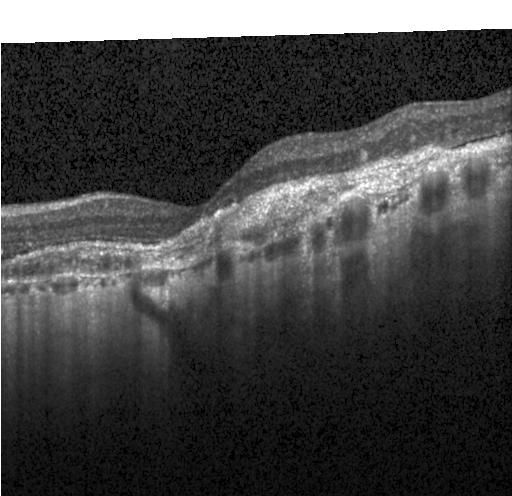 Heidelberg Spectralis OCT system; SD-OCT; retinal OCT B-scan — Diagnosis: choroidal neovascularization (CNV).